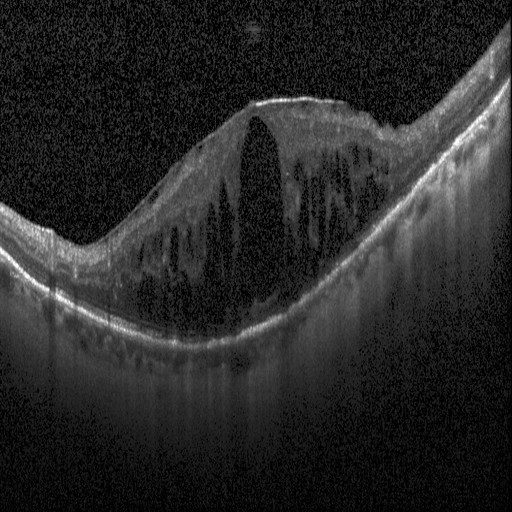 Macular scan. Spectral-domain optical coherence tomography. OCT B-scan. Instrument: Heidelberg Spectralis — OCT finding: diabetic macular edema.